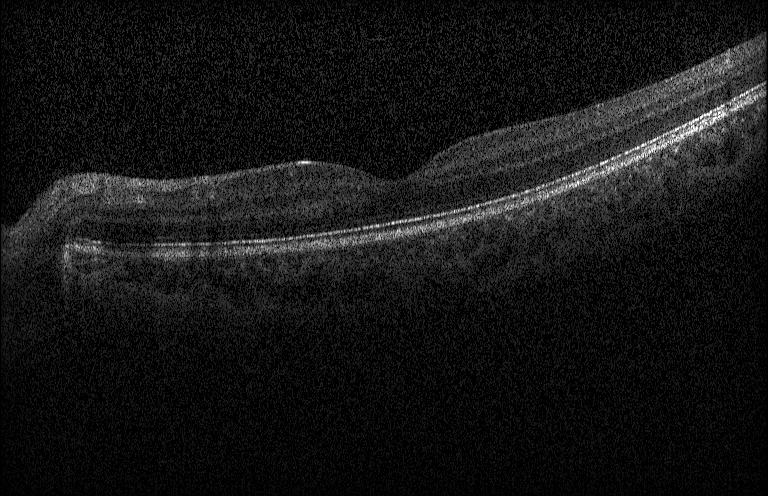

Macular OCT: no choroidal neovascularization, no diabetic macular edema, and no drusen.